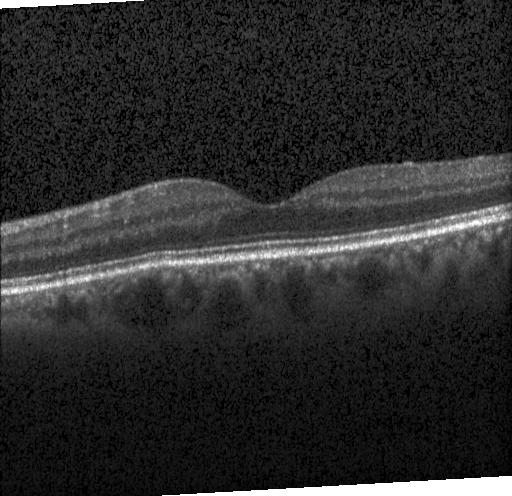 Macular scan, optical coherence tomography scan.
No evidence of CNV, DME, or drusen.